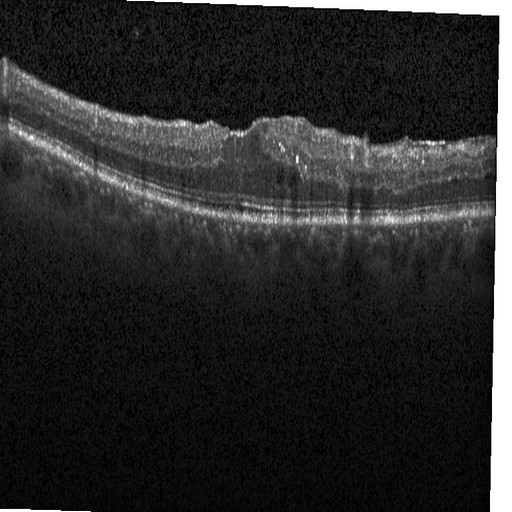
Retinal OCT B-scan — Finding: diabetic macular edema (DME).